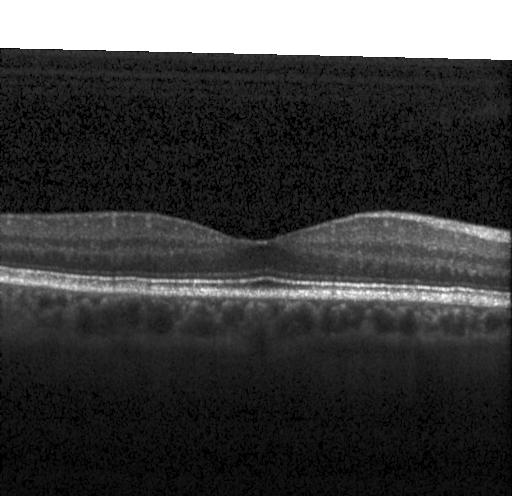 OCT line scan.
Finding: no evidence of choroidal neovascularization, diabetic macular edema, or drusen.